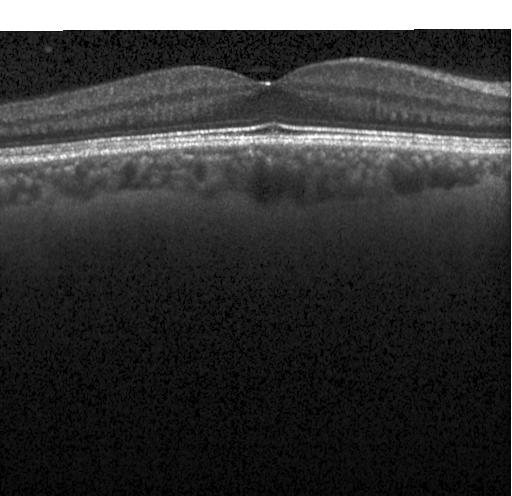 Retinal OCT B-scan · centered on the fovea · Heidelberg Spectralis OCT system. Finding: neither CNV, DME, nor drusen.